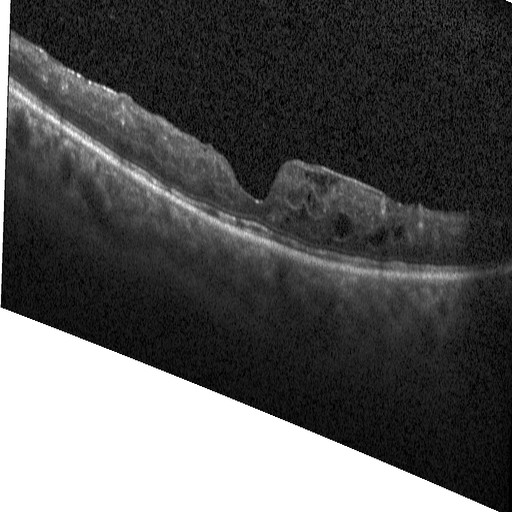 OCT scan showing DME.